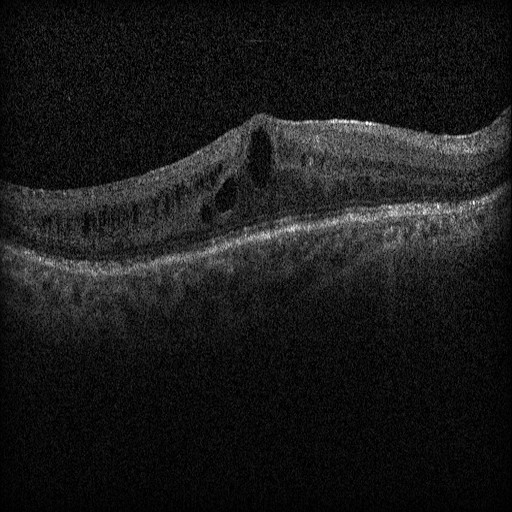

This B-scan demonstrates DME.